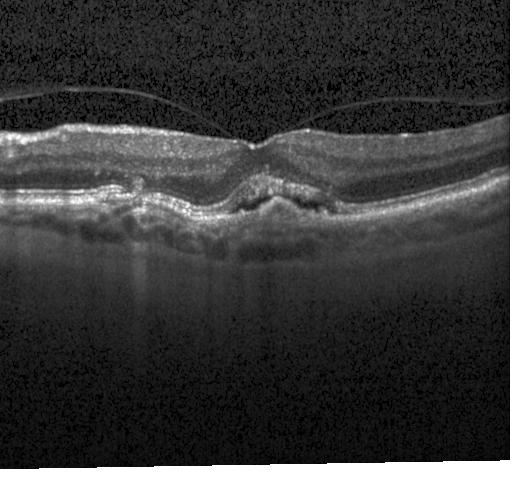 Macular OCT: CNV.